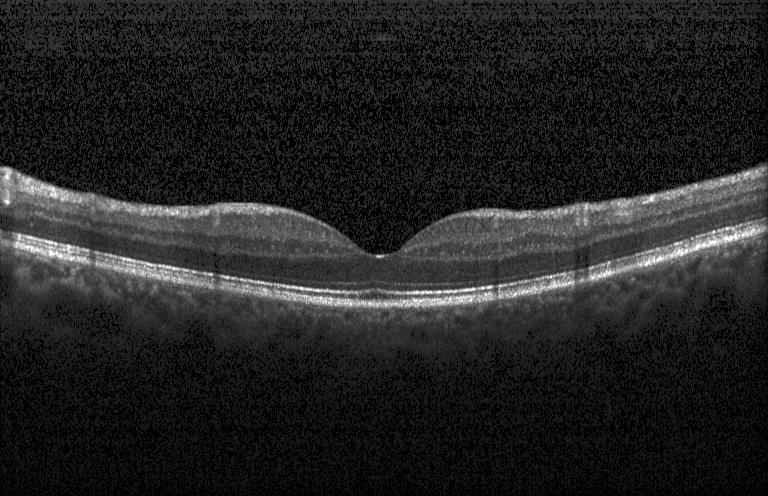
Diagnosis: no choroidal neovascularization, diabetic macular edema, or drusen.